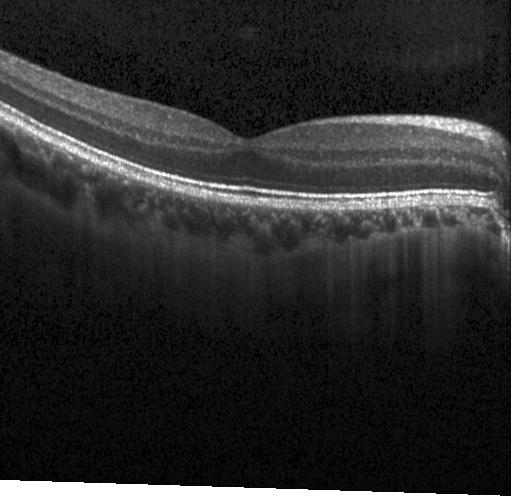
Retinal OCT B-scan; instrument: Heidelberg Spectralis; centered on the fovea; SD-OCT
Macular OCT: neither choroidal neovascularization, diabetic macular edema, nor drusen.